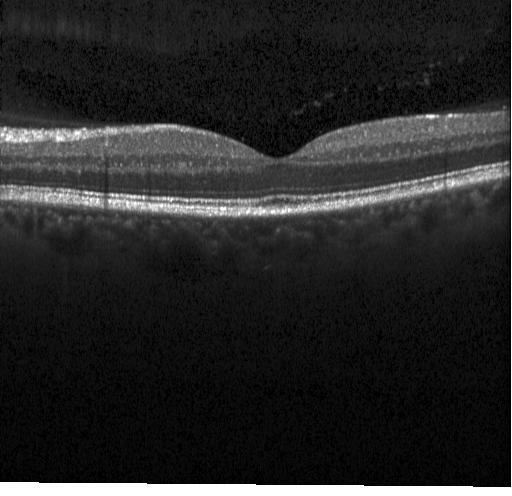
Diagnosis: no evidence of choroidal neovascularization, diabetic macular edema, or drusen.